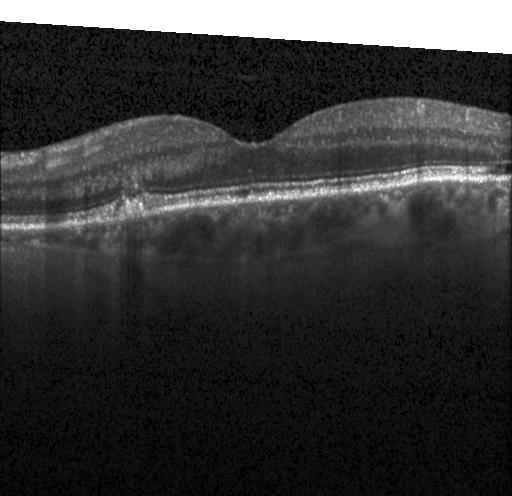

OCT B-scan — Finding: multiple drusen.